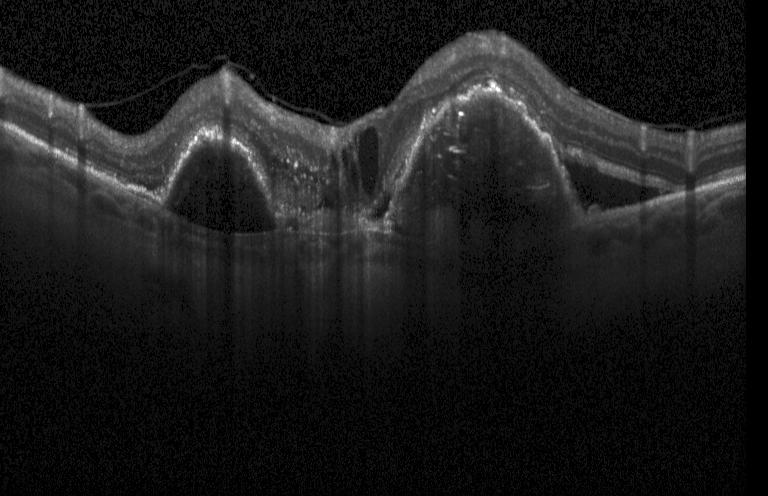

The scan shows CNV.